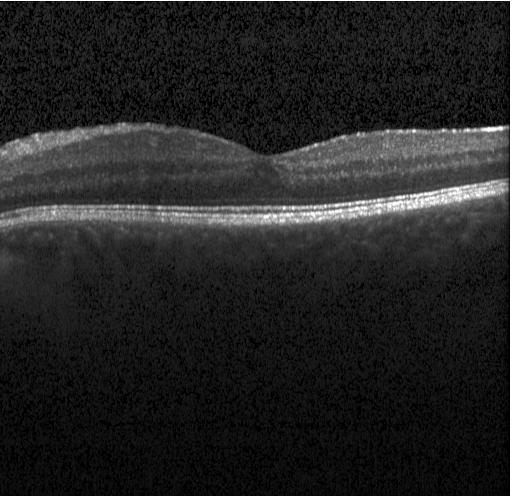
No choroidal neovascularization, no diabetic macular edema, and no drusen.